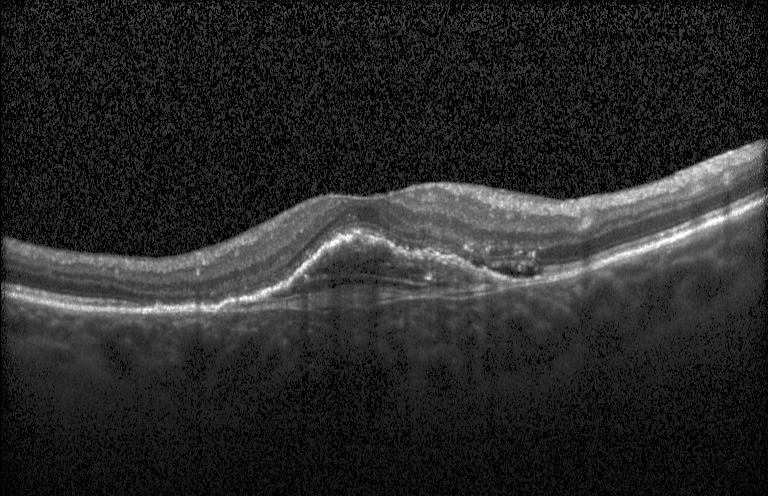 Acquired on a Heidelberg Spectralis, SD-OCT, horizontal scan through the fovea, optical coherence tomography B-scan
Diagnosis: CNV.